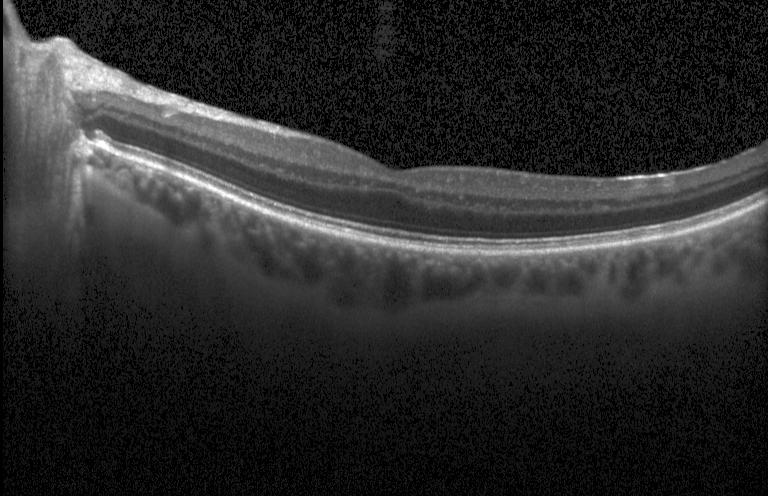
Spectral-domain optical coherence tomography. Heidelberg Spectralis. Centered on the fovea. Retinal OCT B-scan.
OCT finding: no choroidal neovascularization, no diabetic macular edema, and no drusen.